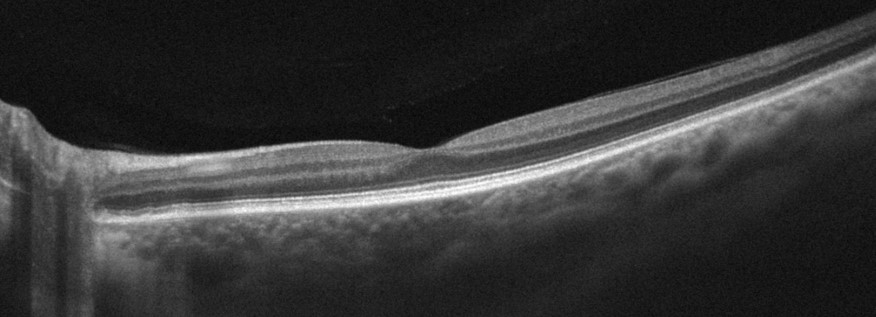 Instrument: Optovue Avanti RTVue XR · retinal OCT cross-section.
Dx: no AMD, DME, ERM, RAO, RVO, or VID.